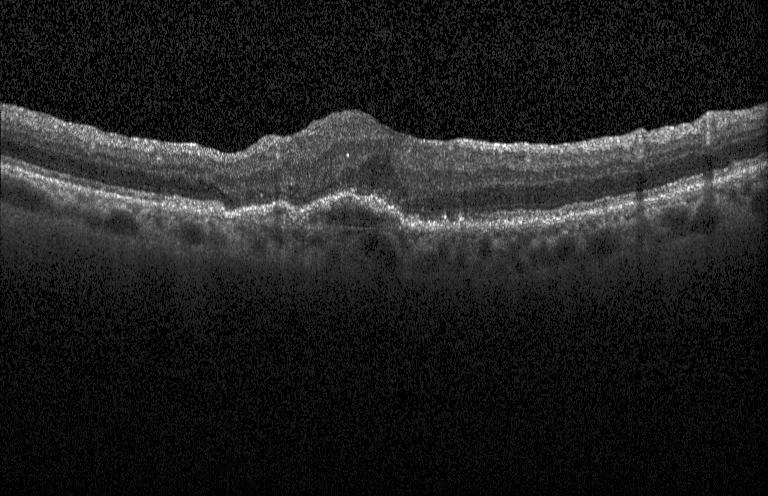 Optical coherence tomography B-scan
Finding: a choroidal neovascular membrane.